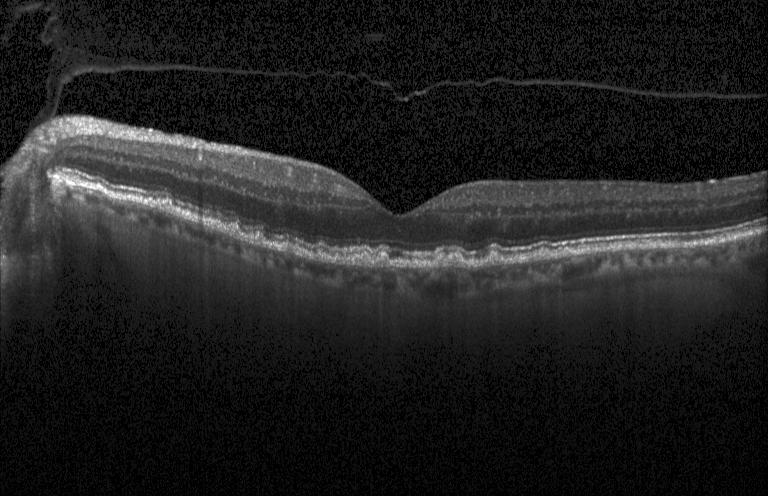

Impression: sub-RPE drusenoid deposits.